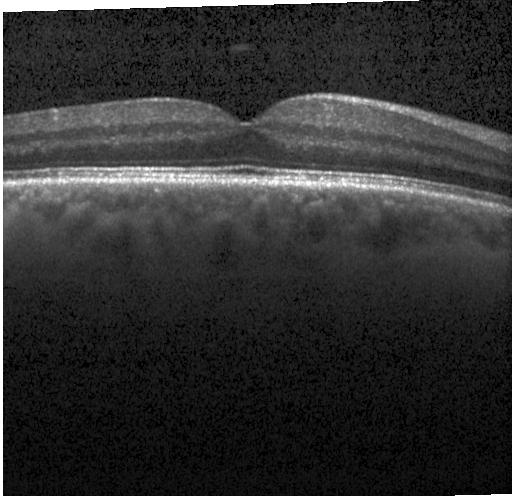

Acquired on a Heidelberg Spectralis, SD-OCT, horizontal scan through the fovea, optical coherence tomography B-scan. Impression: no choroidal neovascularization, no diabetic macular edema, and no drusen.